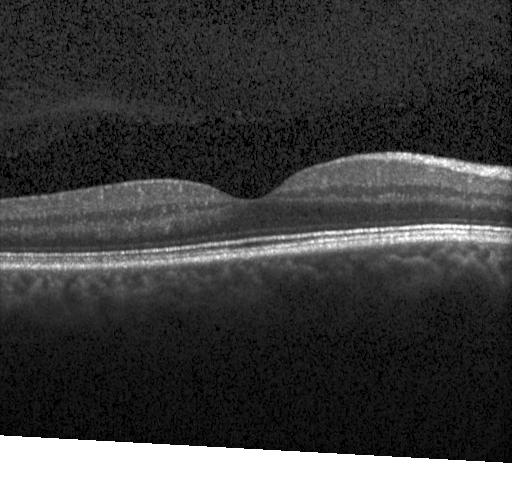

OCT scan showing no choroidal neovascularization, diabetic macular edema, or drusen.